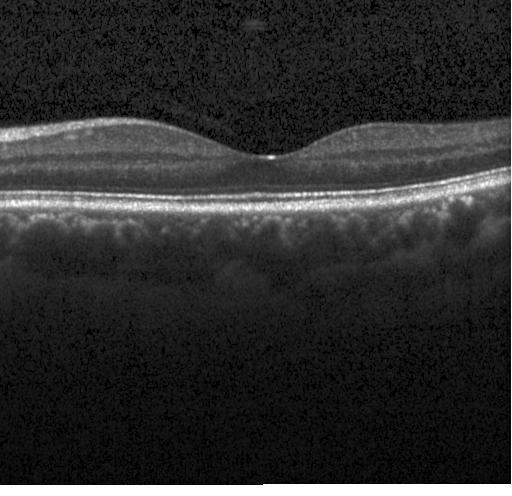

Retinal OCT cross-section
Diagnosis: no choroidal neovascularization, diabetic macular edema, or drusen.